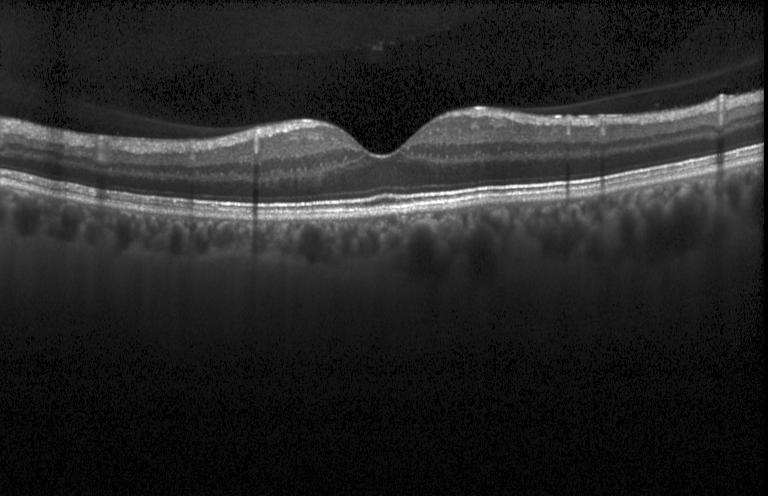 Optical coherence tomography B-scan. Diagnosis: no evidence of choroidal neovascularization, diabetic macular edema, or drusen.